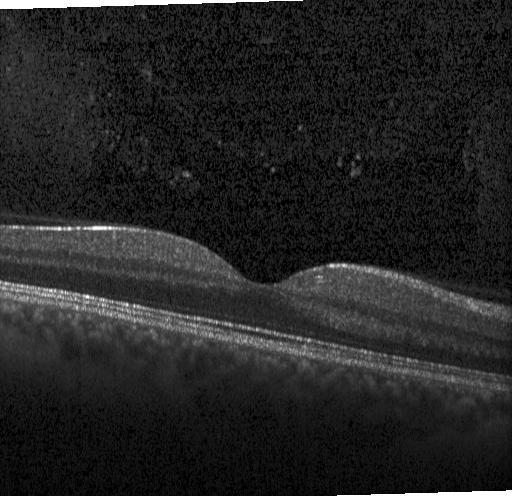 Acquired on a Heidelberg Spectralis, OCT line scan, centered on the fovea, SD-OCT — Diagnosis: neither CNV, DME, nor drusen.